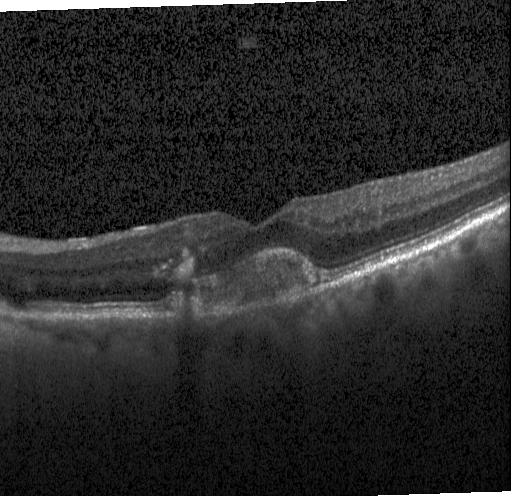

Macular scan; instrument: Heidelberg Spectralis; retinal OCT B-scan
Impression: choroidal neovascularization.